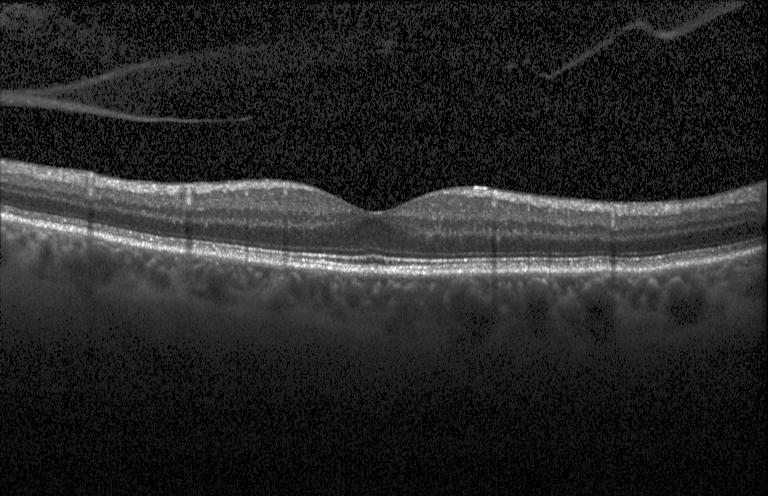

Retinal OCT cross-section; spectral-domain OCT; Heidelberg Spectralis OCT system; horizontal scan through the fovea. The scan shows no evidence of choroidal neovascularization, diabetic macular edema, or drusen.